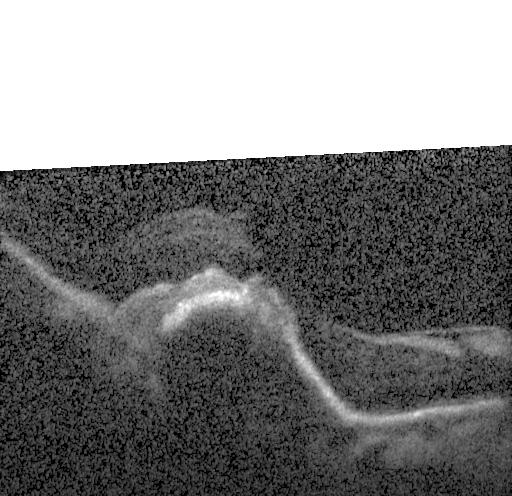
Spectral-domain optical coherence tomography, optical coherence tomography scan — Dx: choroidal neovascularization (CNV).